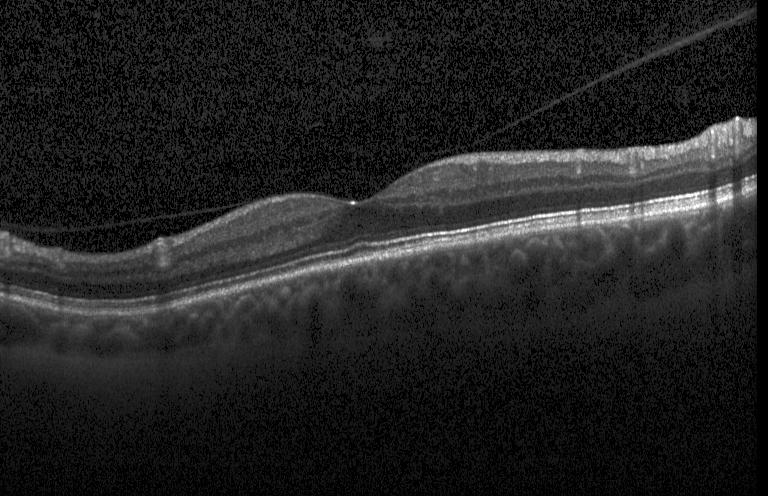
No evidence of choroidal neovascularization, diabetic macular edema, or drusen.